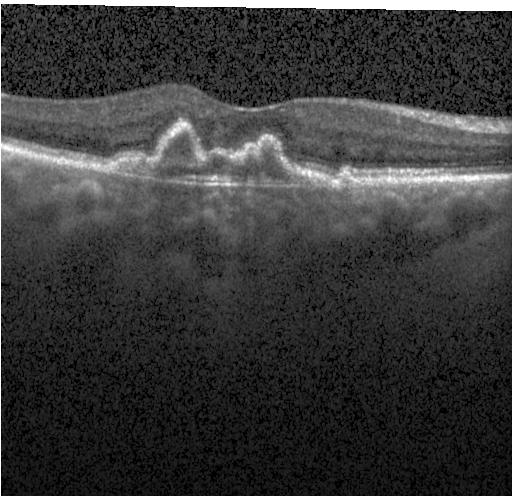
Macular OCT: a choroidal neovascular membrane.